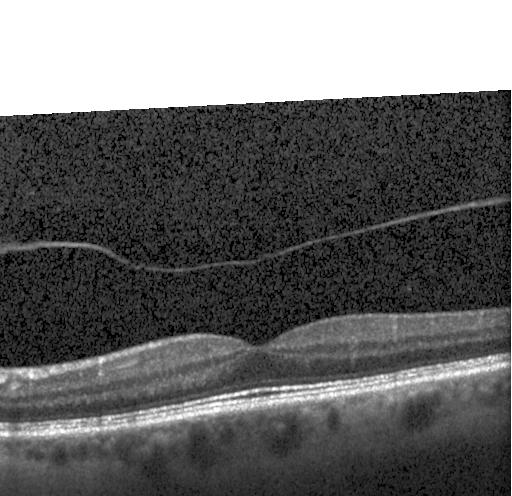
OCT B-scan.
Finding: neither choroidal neovascularization, diabetic macular edema, nor drusen.